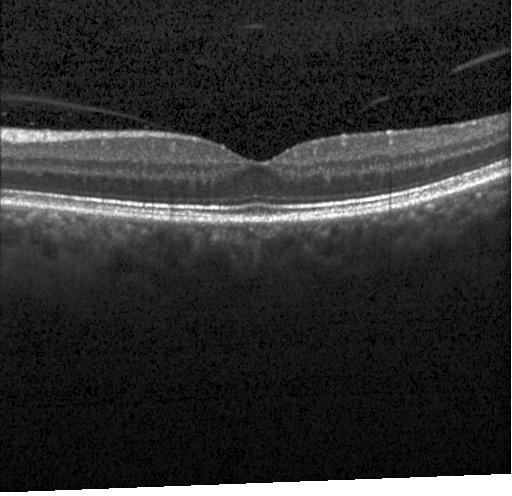
Horizontal scan through the fovea · optical coherence tomography B-scan · instrument: Heidelberg Spectralis.
OCT finding: no evidence of choroidal neovascularization, diabetic macular edema, or drusen.